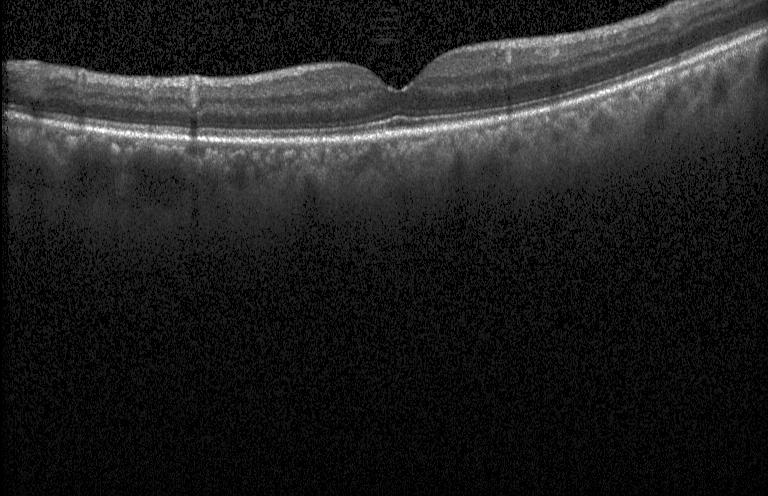

Heidelberg Spectralis. Through the macula. Retinal OCT cross-section. Spectral-domain OCT
OCT finding: neither CNV, DME, nor drusen.